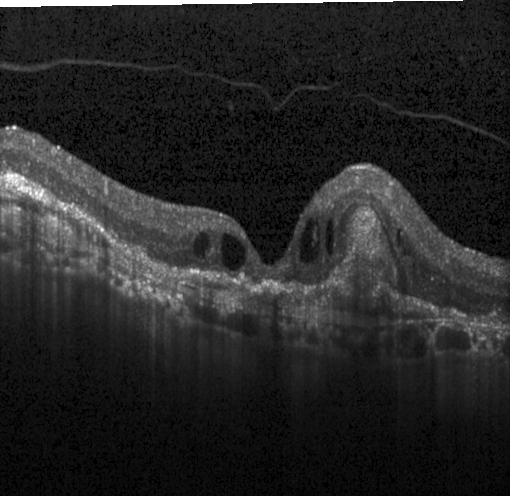 Optical coherence tomography B-scan · through the macula · acquired on a Heidelberg Spectralis · SD-OCT
This B-scan demonstrates CNV.